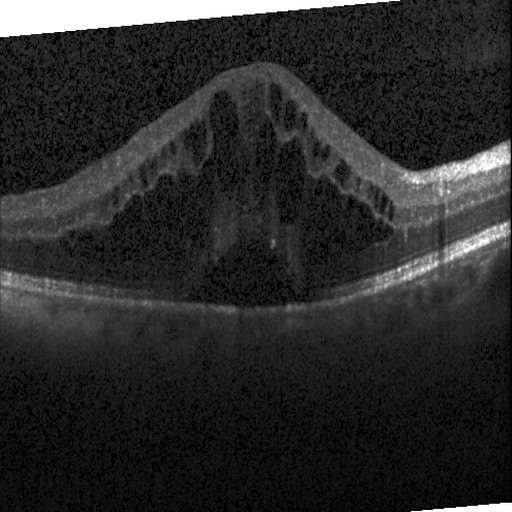

OCT finding: diabetic macular edema (DME).